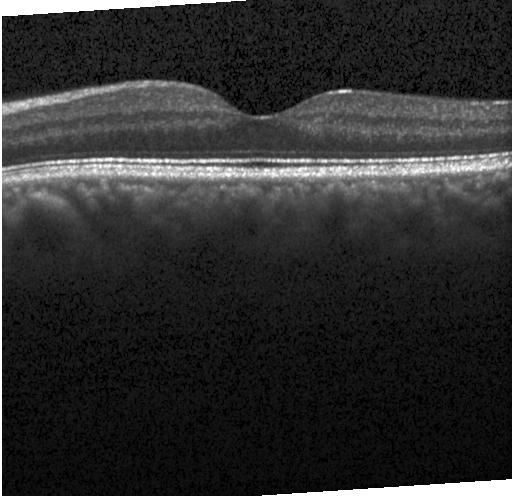
Spectral-domain OCT · Heidelberg Spectralis · horizontal scan through the fovea · retinal OCT B-scan. Diagnosis: no choroidal neovascularization, no diabetic macular edema, and no drusen.